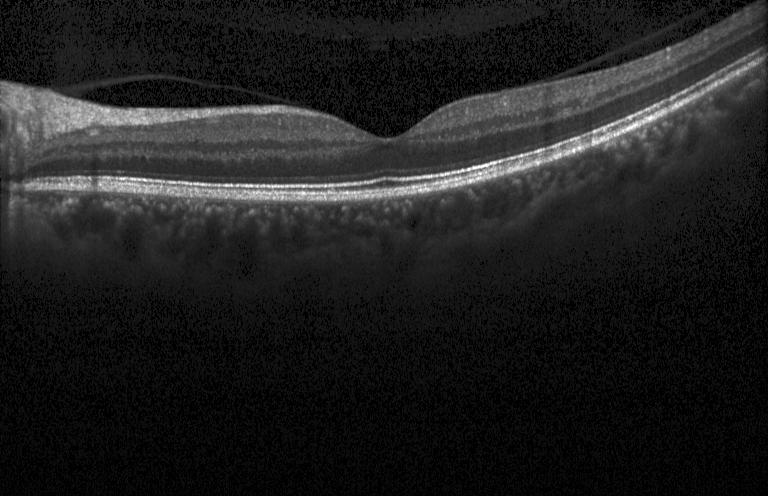
Spectral-domain optical coherence tomography; OCT line scan — Macular OCT: no choroidal neovascularization, diabetic macular edema, or drusen.